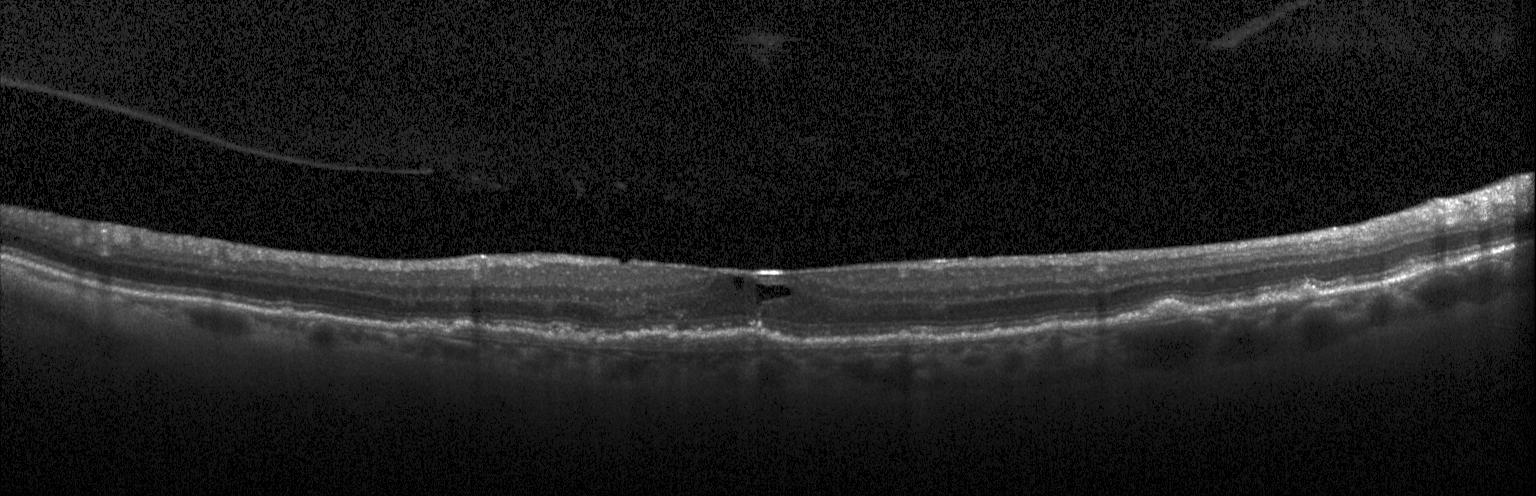 Macular scan; OCT B-scan
Finding: CNV.